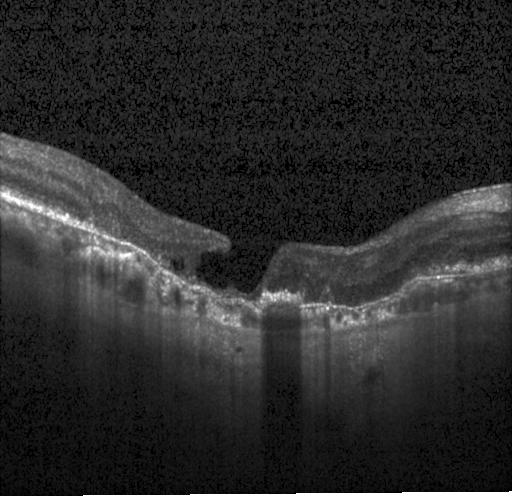

Diagnosis: a choroidal neovascular membrane.